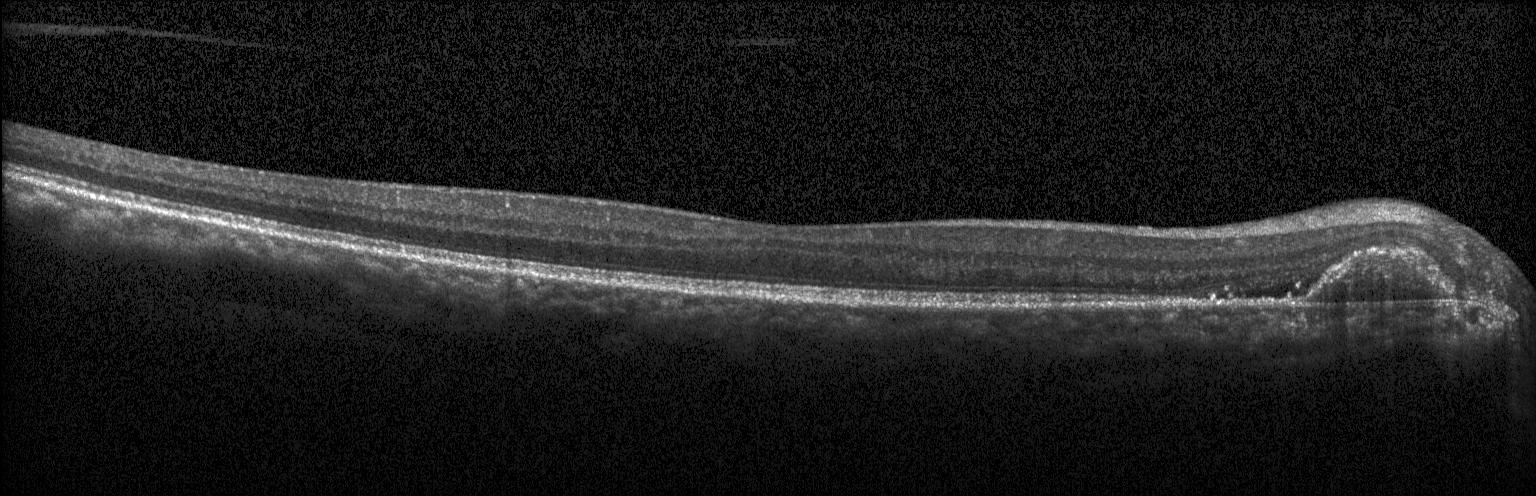
Retinal OCT cross-section showing CNV.